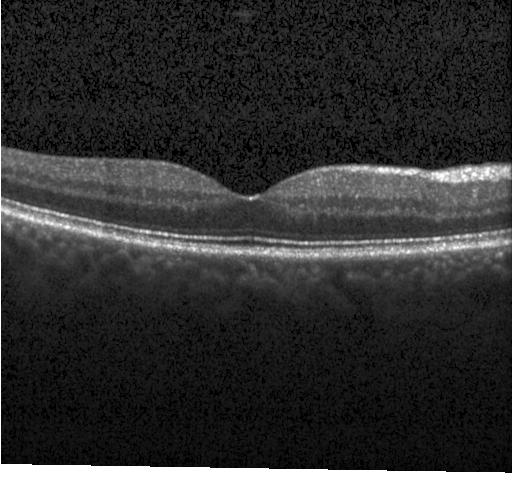

Horizontal scan through the fovea, Heidelberg Spectralis OCT system, OCT line scan, spectral-domain OCT
Finding: neither choroidal neovascularization, diabetic macular edema, nor drusen.